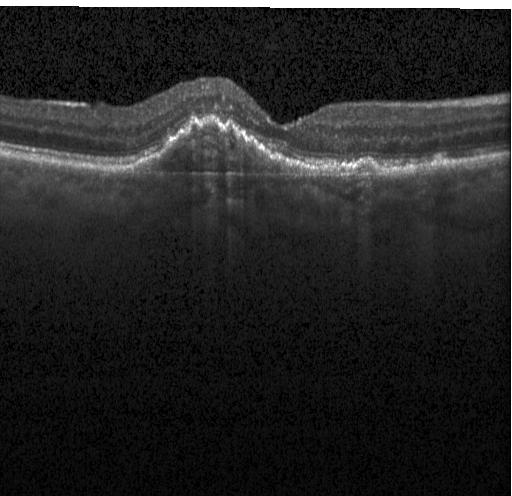
Through the macula. Retinal OCT B-scan.
Choroidal neovascularization.